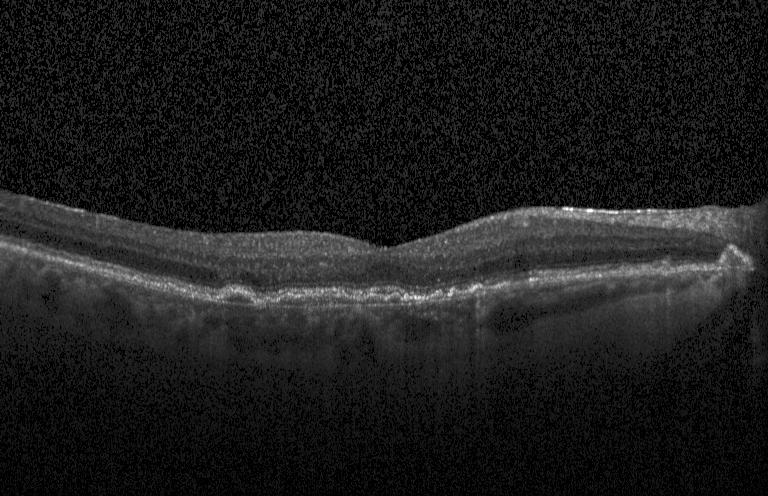

Finding: choroidal neovascularization (CNV).